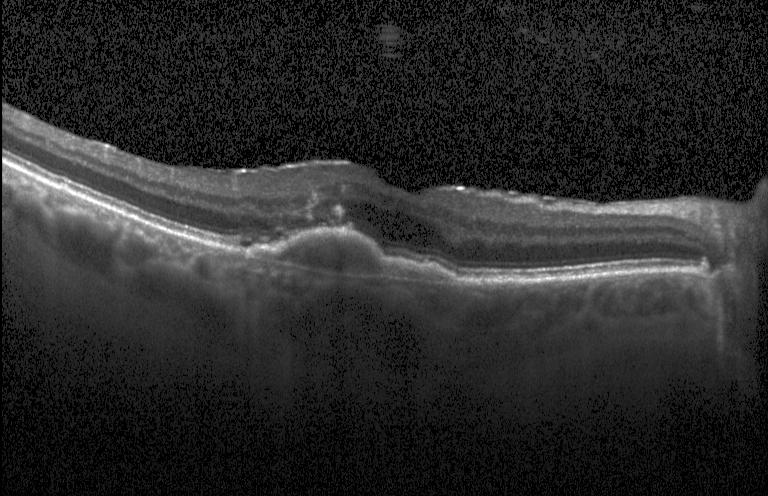 Heidelberg Spectralis OCT system. OCT line scan. Finding: a choroidal neovascular membrane.